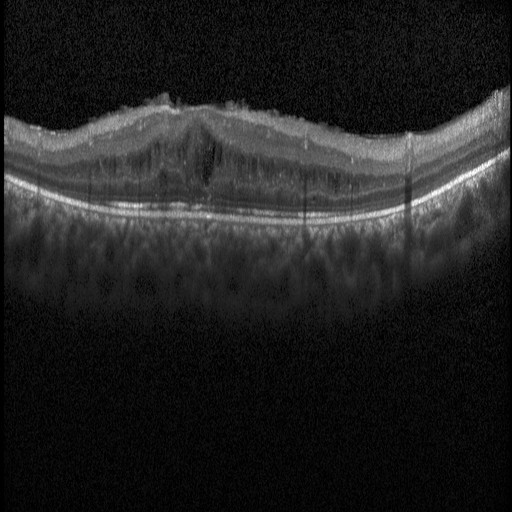

Impression: DME.